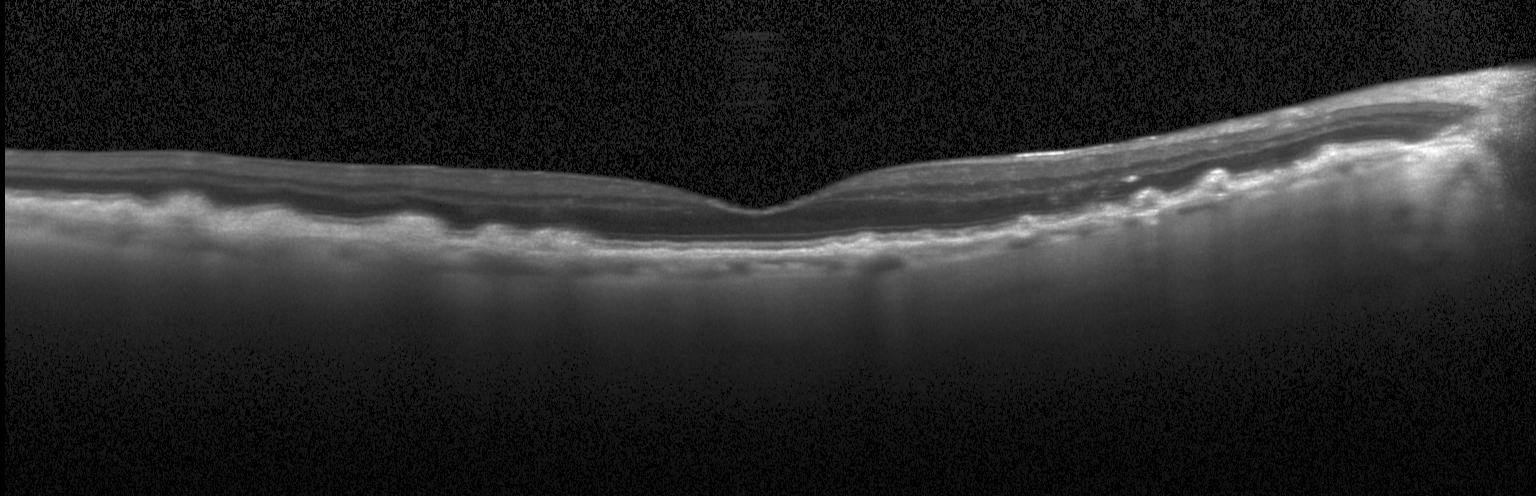 Acquired on a Heidelberg Spectralis · OCT line scan — Diagnosis: multiple drusen.